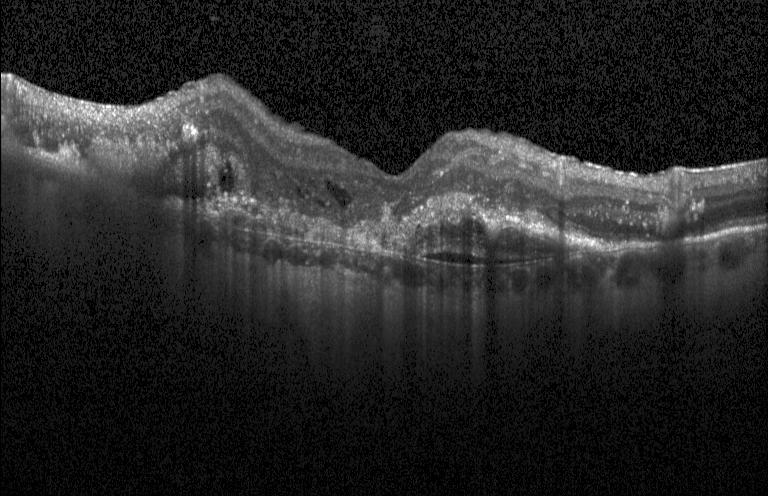 Retinal OCT cross-section showing a choroidal neovascular membrane.